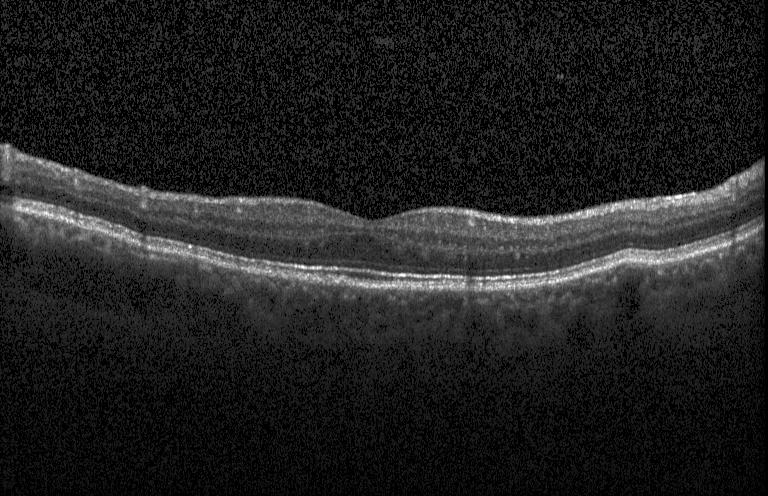 Optical coherence tomography B-scan, horizontal scan through the fovea, spectral-domain OCT, Heidelberg Spectralis — Finding: no choroidal neovascularization, no diabetic macular edema, and no drusen.